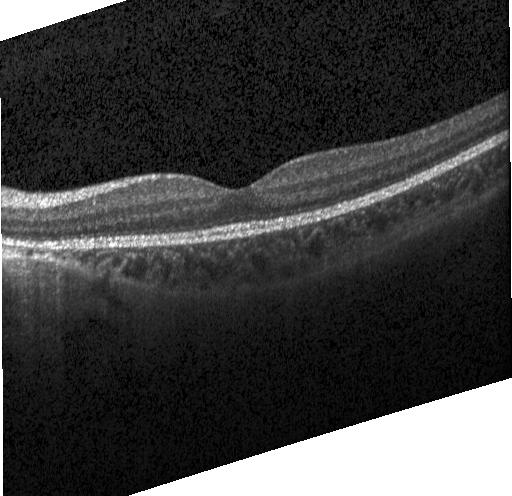 Optical coherence tomography scan. Impression: no choroidal neovascularization, diabetic macular edema, or drusen.